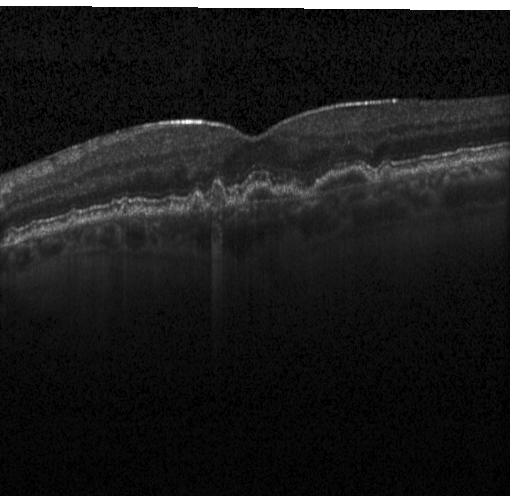 Impression: sub-RPE drusenoid deposits.